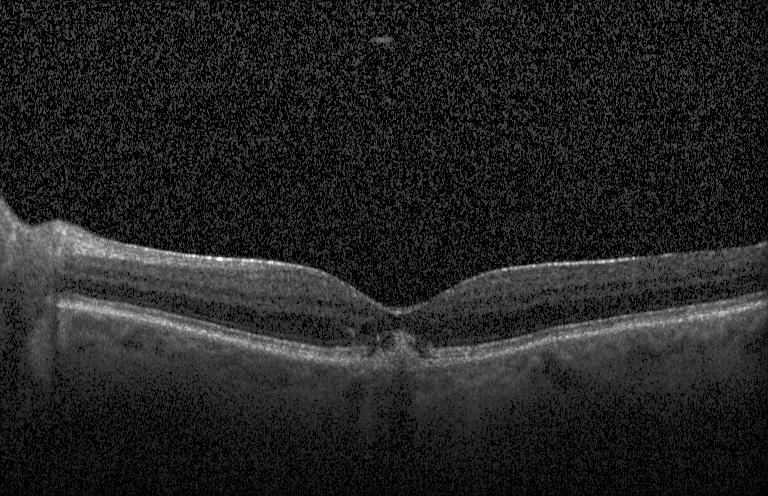 Spectral-domain optical coherence tomography. Retinal OCT B-scan. OCT finding: a choroidal neovascular membrane.